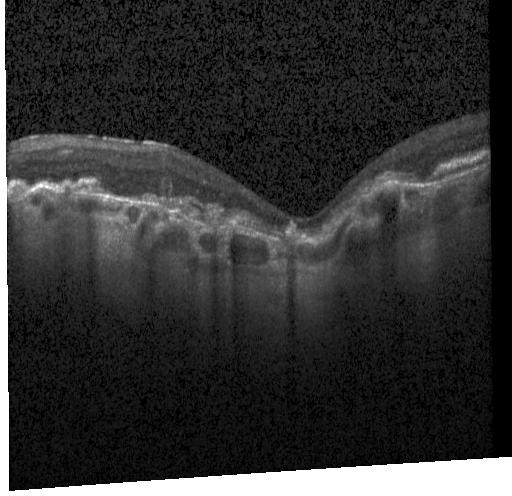

Retinal OCT cross-section · centered on the fovea · acquired on a Heidelberg Spectralis.
Diagnosis: a choroidal neovascular membrane.